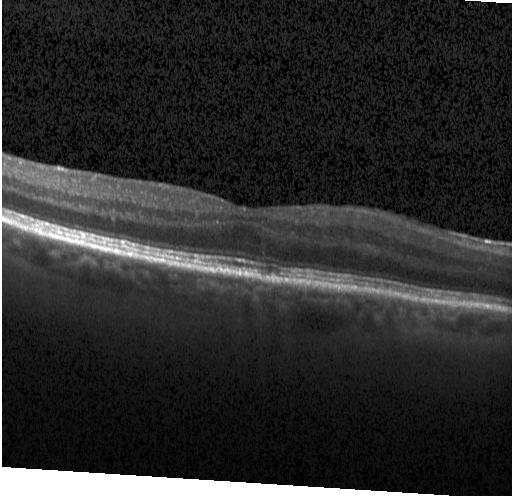 Centered on the fovea · OCT line scan · spectral-domain OCT
Macular OCT: neither choroidal neovascularization, diabetic macular edema, nor drusen.